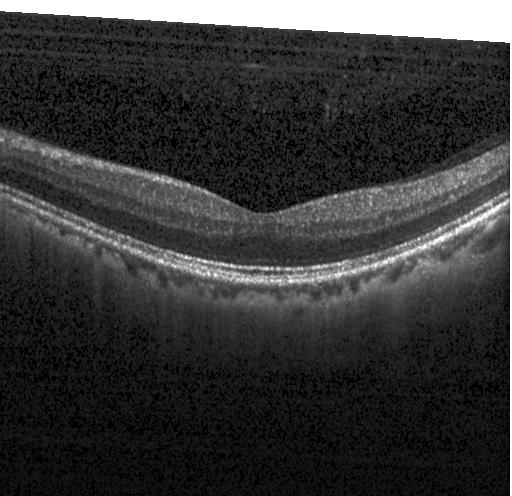
Macular OCT: no choroidal neovascularization, diabetic macular edema, or drusen.